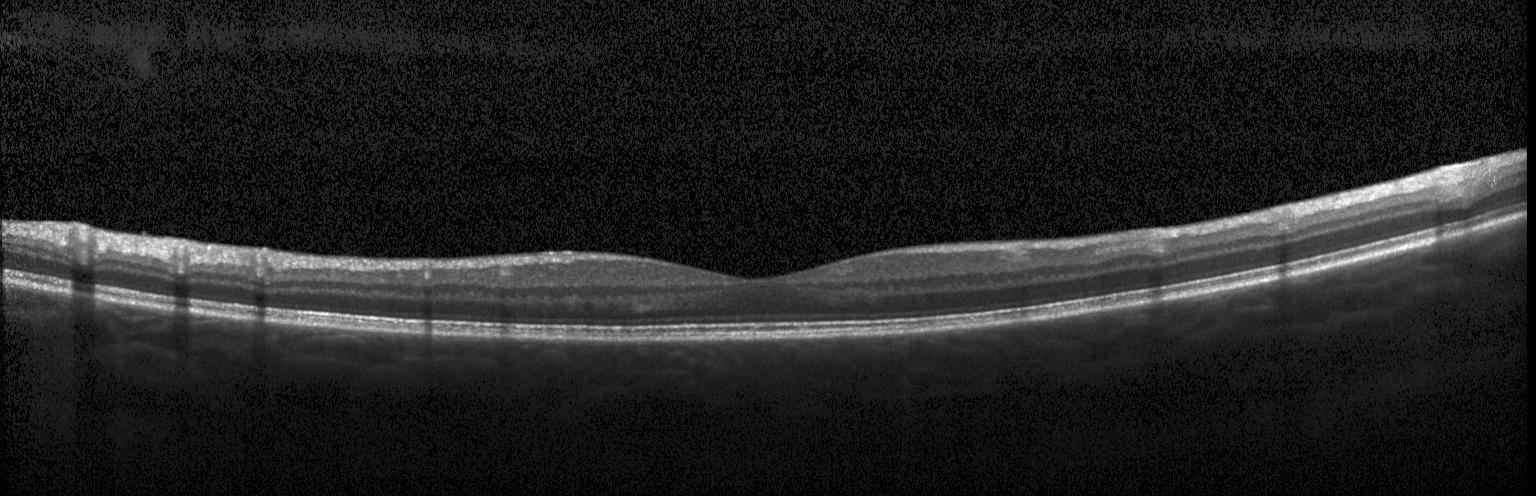 Retinal OCT cross-section, horizontal scan through the fovea, spectral-domain optical coherence tomography
Impression: no CNV, DME, or drusen.